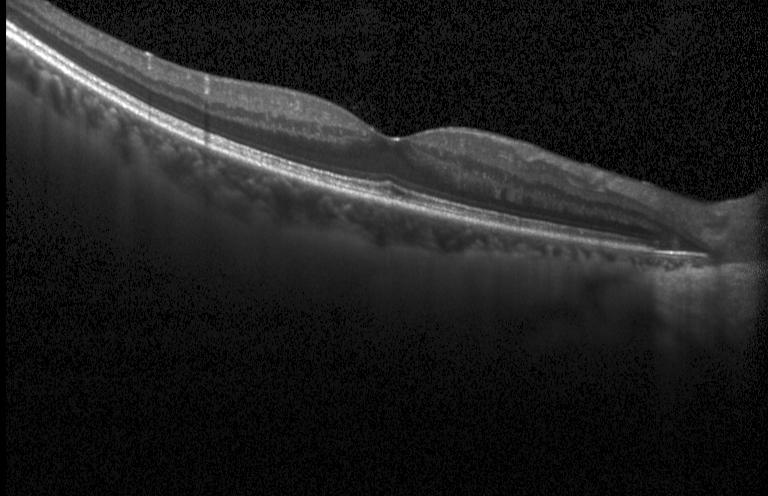 OCT B-scan. SD-OCT — Finding: no CNV, no DME, and no drusen.